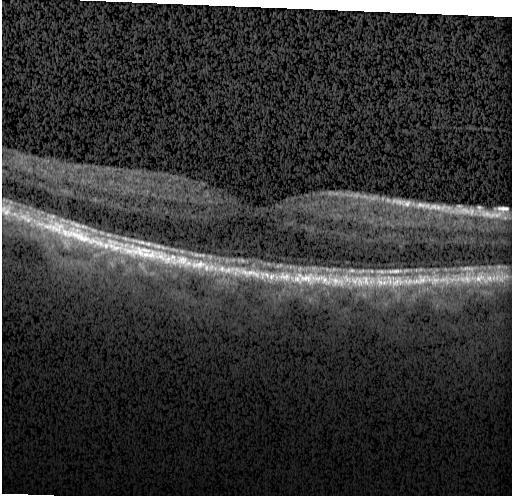 Heidelberg Spectralis · SD-OCT · OCT line scan.
Diagnosis: no choroidal neovascularization, no diabetic macular edema, and no drusen.